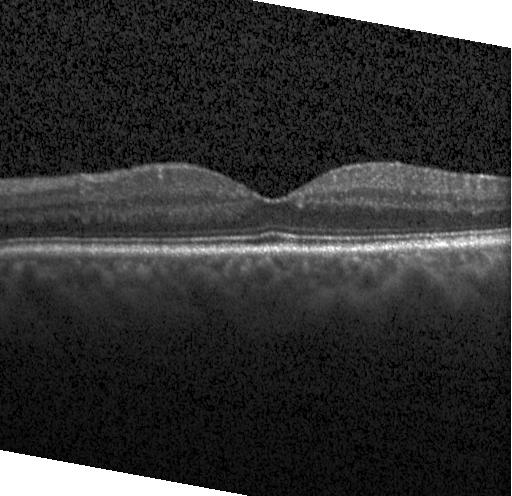
Optical coherence tomography B-scan · acquired on a Heidelberg Spectralis. This B-scan demonstrates no choroidal neovascularization, diabetic macular edema, or drusen.